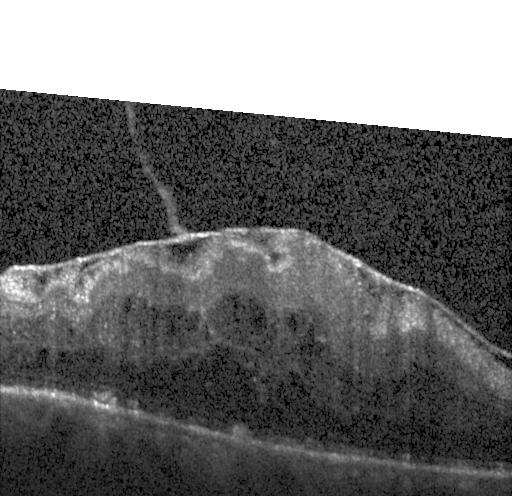
Acquired on a Heidelberg Spectralis; retinal OCT B-scan
Assessment: diabetic macular edema.